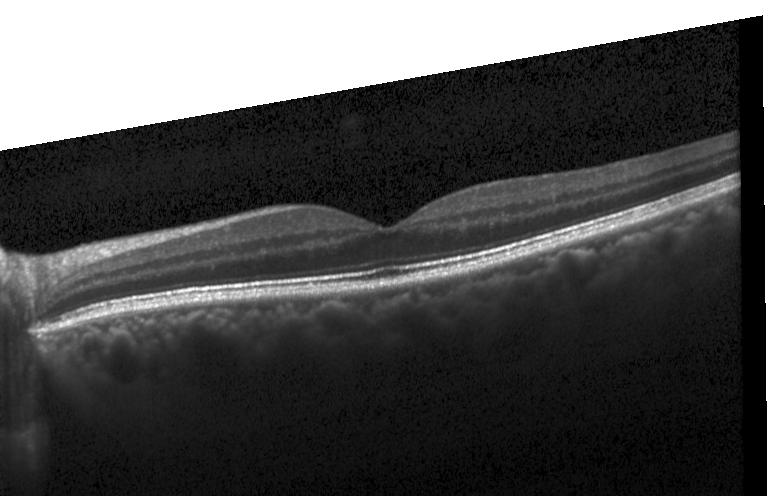
Optical coherence tomography scan. Spectral-domain optical coherence tomography. Heidelberg Spectralis. Finding: no evidence of choroidal neovascularization, diabetic macular edema, or drusen.